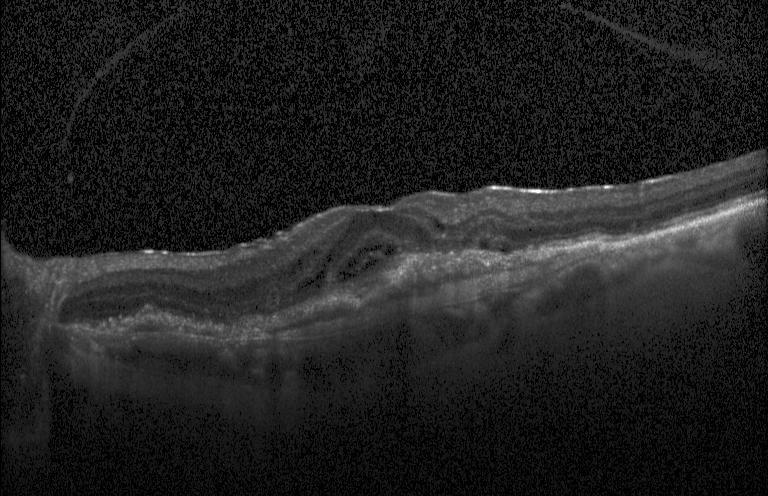
OCT B-scan; horizontal scan through the fovea. Dx: a choroidal neovascular membrane.